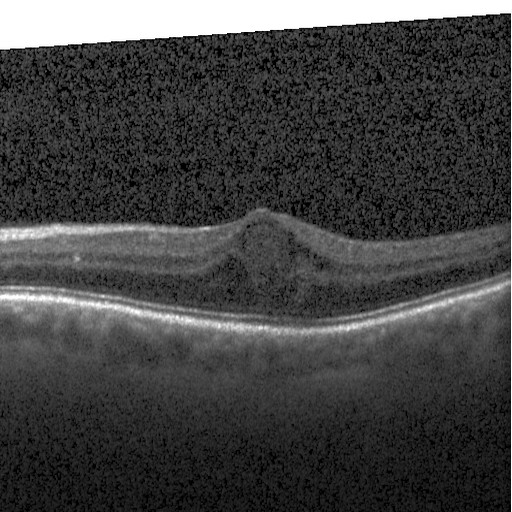
Horizontal scan through the fovea. Retinal OCT cross-section — Assessment: diabetic macular edema.